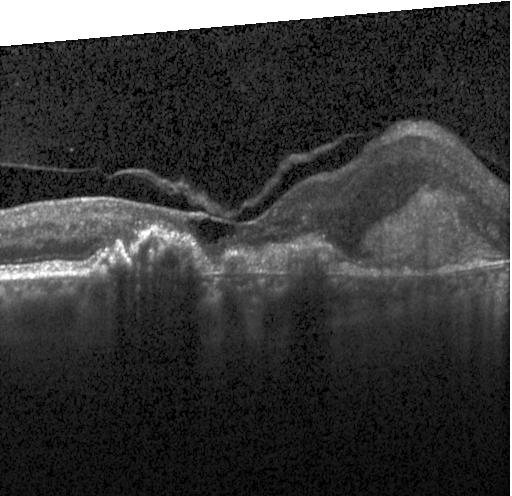
Assessment: a choroidal neovascular membrane.